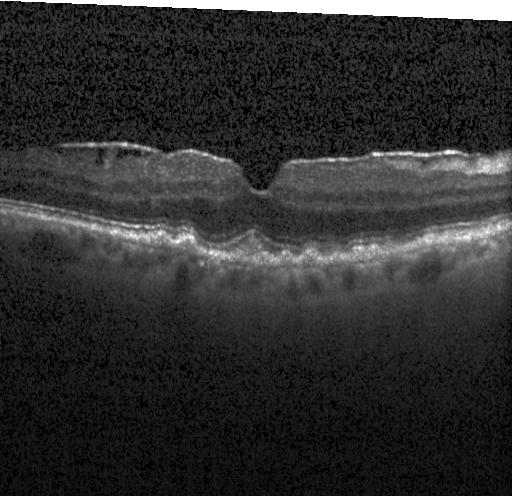 Spectral-domain OCT B-scan: multiple drusen.